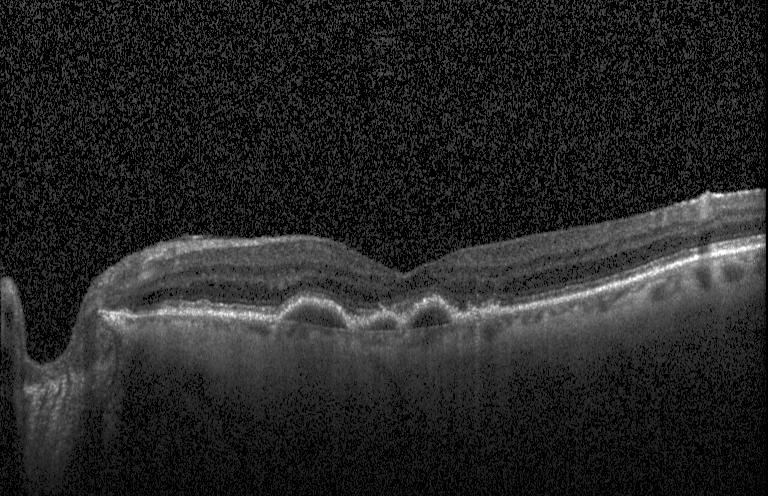 OCT B-scan, spectral-domain OCT, through the macula, acquired on a Heidelberg Spectralis. Assessment: choroidal neovascularization (CNV).